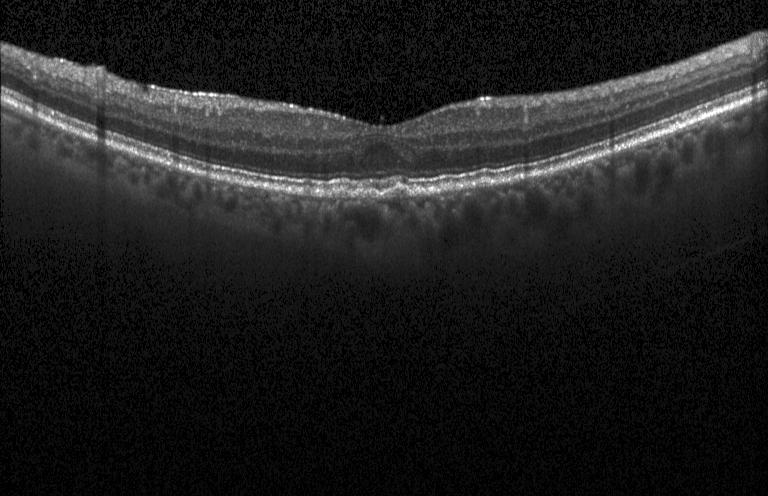

Optical coherence tomography B-scan
This B-scan demonstrates drusen.